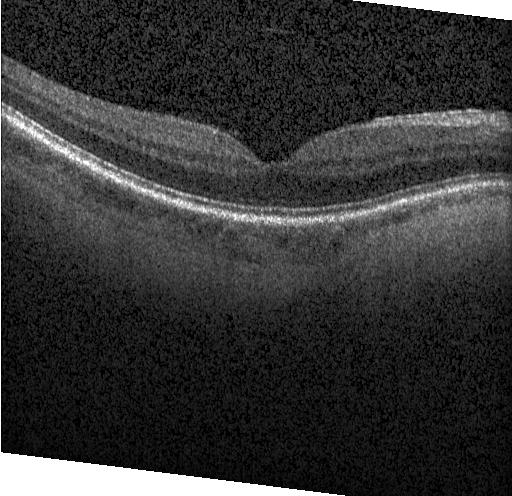
Optical coherence tomography scan.
The scan shows no choroidal neovascularization, no diabetic macular edema, and no drusen.